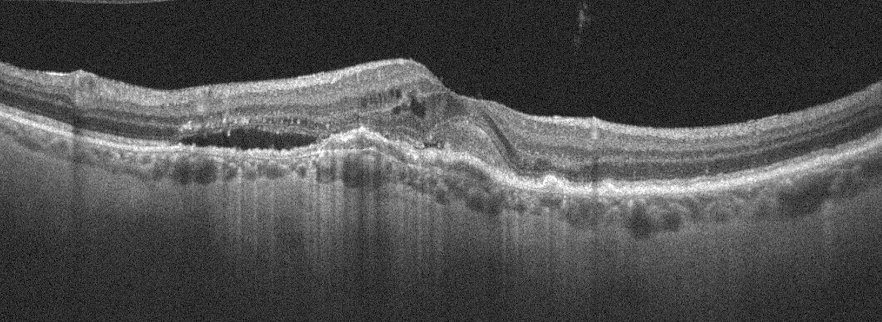
Retinal OCT cross-section showing age-related macular degeneration.